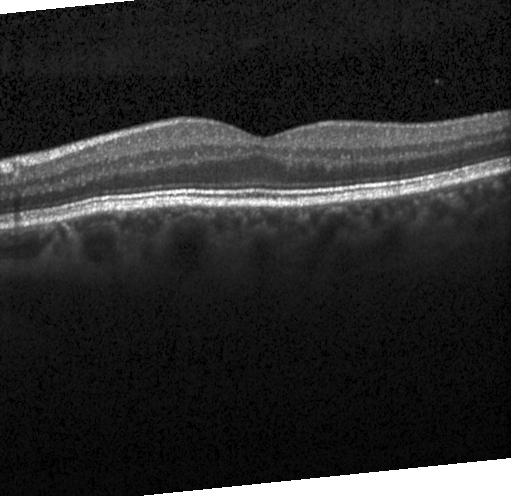 Retinal OCT B-scan.
Impression: no CNV, DME, or drusen.